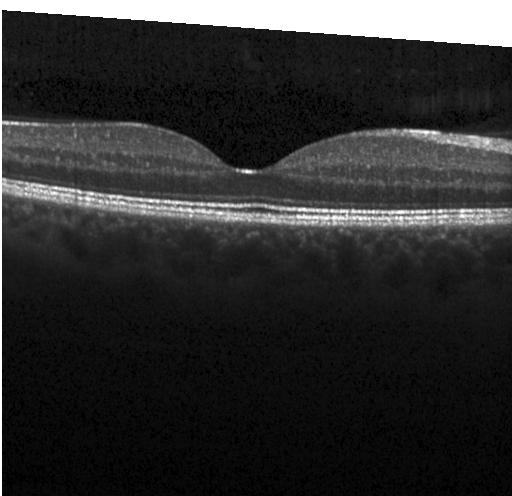 Diagnosis: neither choroidal neovascularization, diabetic macular edema, nor drusen.